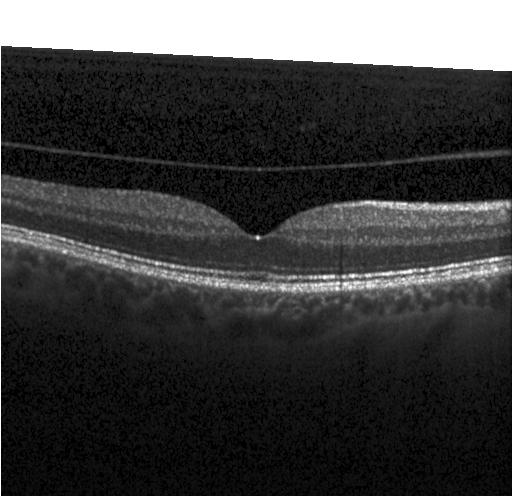
Assessment: neither choroidal neovascularization, diabetic macular edema, nor drusen.